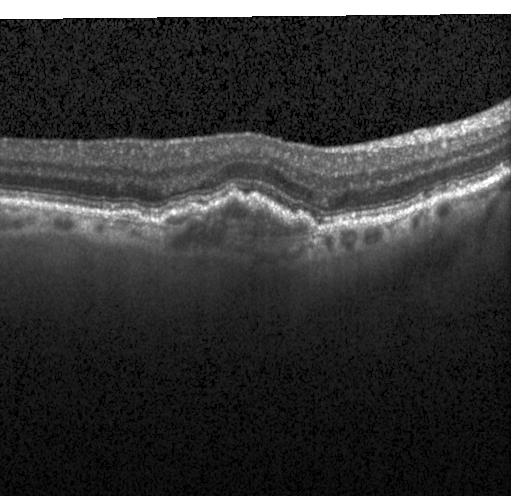
Spectral-domain optical coherence tomography · centered on the fovea · Heidelberg Spectralis · OCT B-scan.
OCT finding: choroidal neovascularization (CNV).